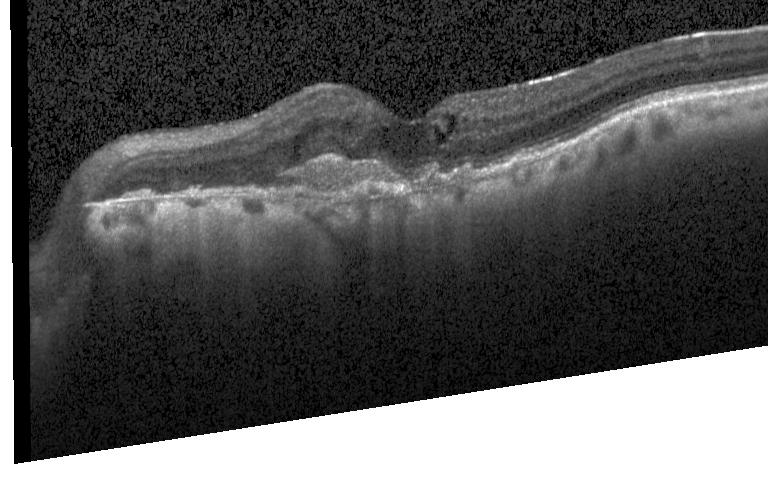
Retinal OCT B-scan — Finding: a choroidal neovascular membrane.